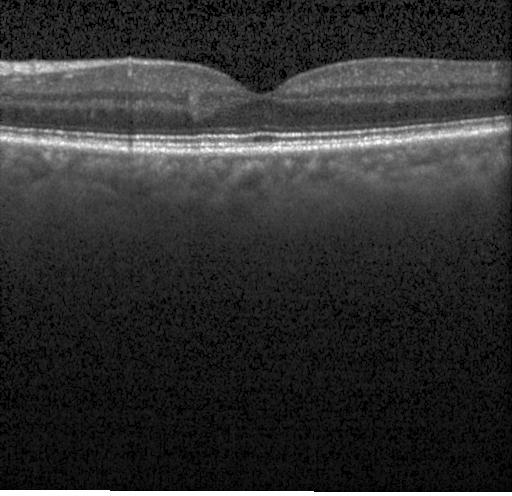
Dx: no CNV, DME, or drusen.